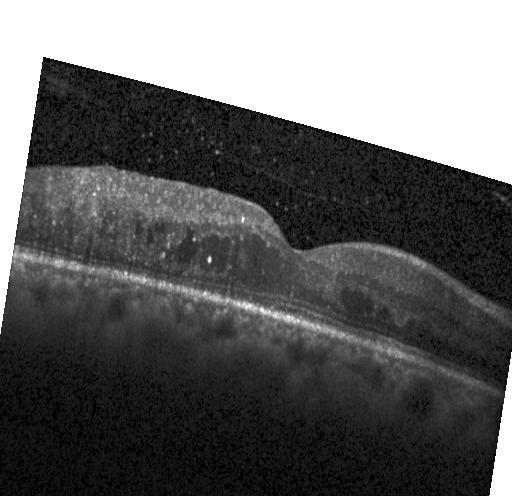
Assessment: diabetic macular edema.